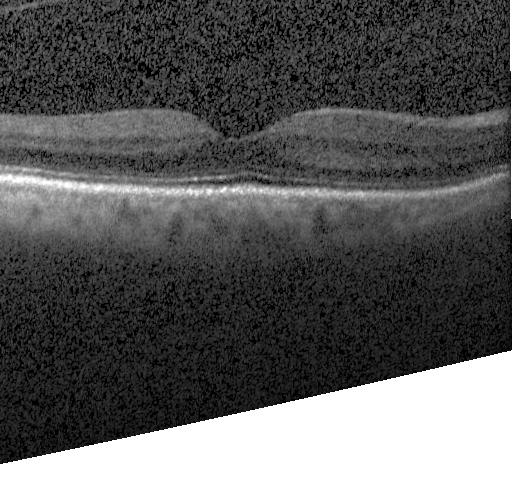

SD-OCT; retinal OCT B-scan. Impression: no CNV, DME, or drusen.